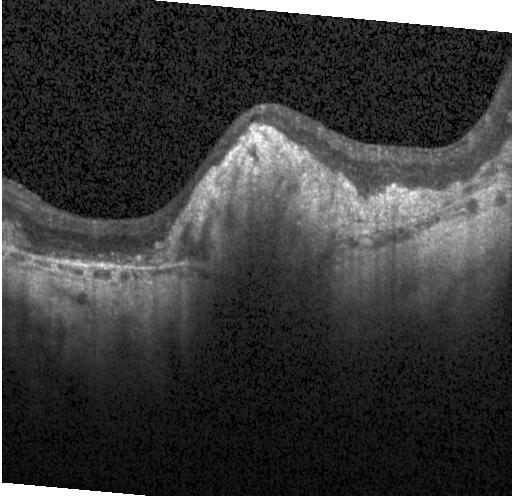

Spectral-domain optical coherence tomography · Heidelberg Spectralis · retinal OCT cross-section. Impression: choroidal neovascularization (CNV).